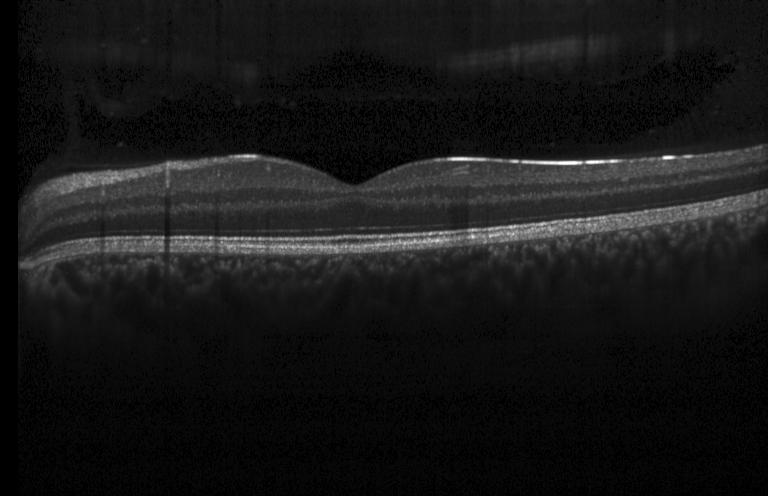
Spectral-domain OCT; through the macula; Heidelberg Spectralis OCT system; optical coherence tomography scan — Diagnosis: neither CNV, DME, nor drusen.